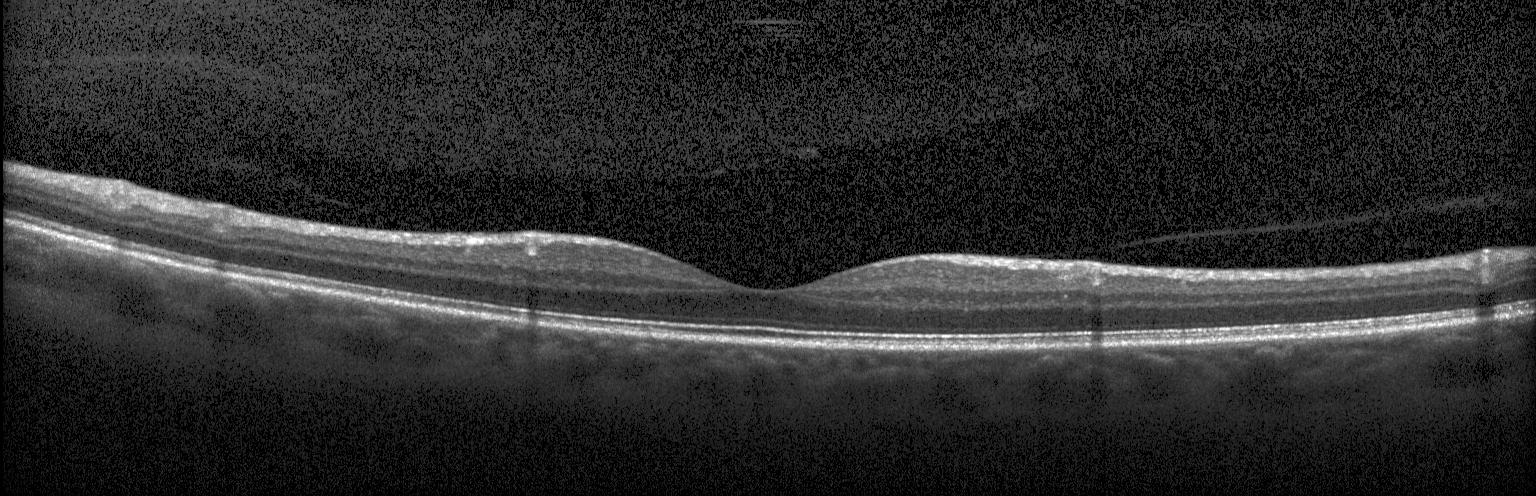
This B-scan demonstrates no choroidal neovascularization, diabetic macular edema, or drusen.